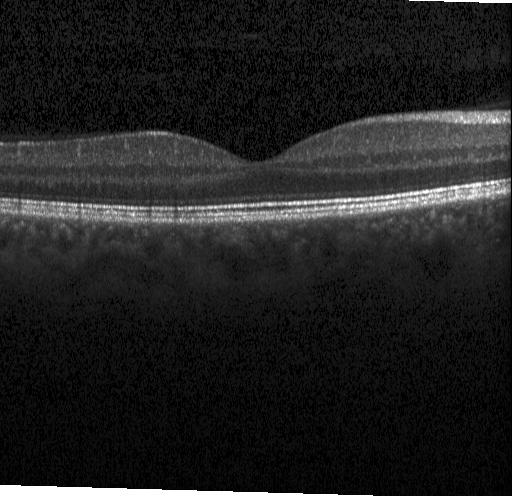 Acquired on a Heidelberg Spectralis, OCT line scan
Macular OCT: no choroidal neovascularization, no diabetic macular edema, and no drusen.